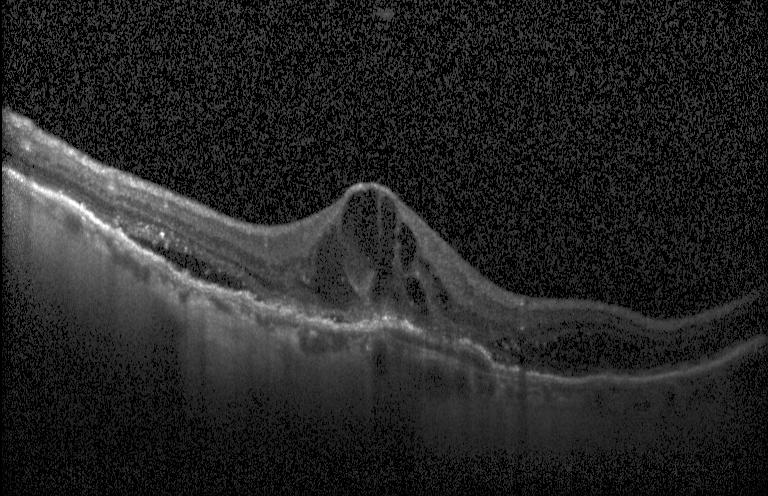
Dx: choroidal neovascularization.